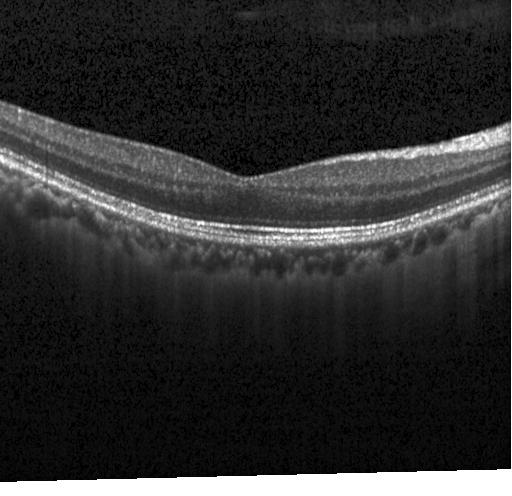 Fovea-centered; Heidelberg Spectralis OCT system; SD-OCT; OCT B-scan
Finding: no evidence of choroidal neovascularization, diabetic macular edema, or drusen.